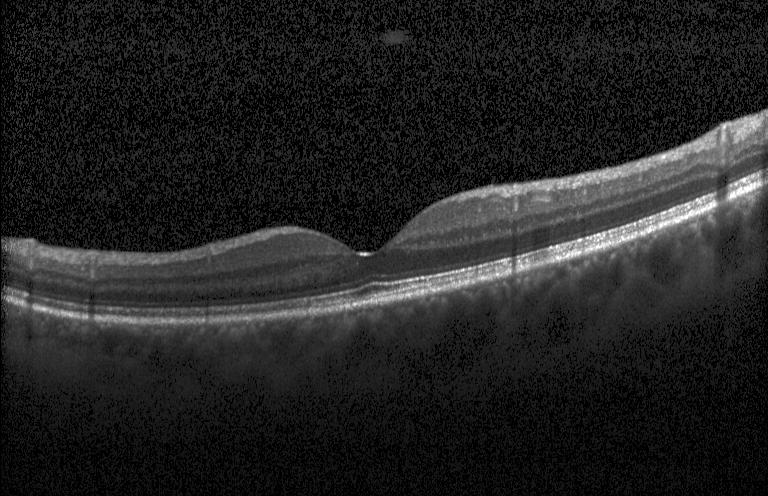 OCT B-scan showing no evidence of choroidal neovascularization, diabetic macular edema, or drusen.